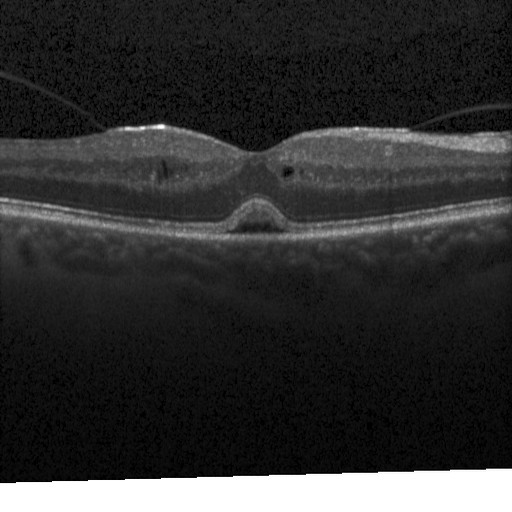

Optical coherence tomography scan. Diabetic macular edema.